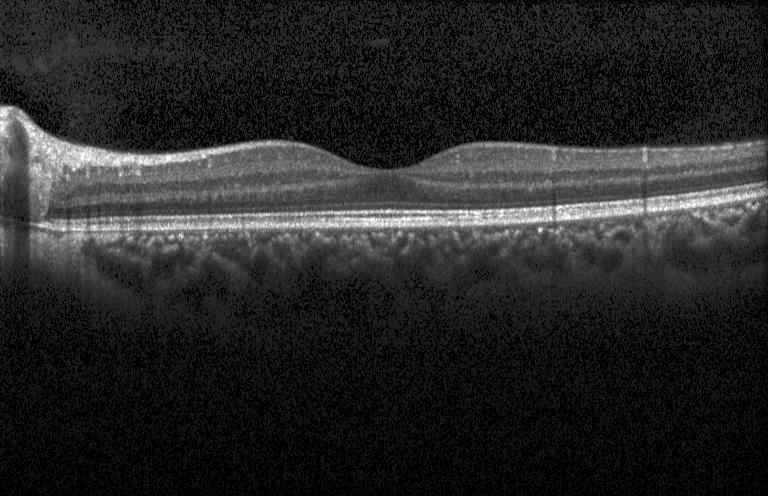 Fovea-centered. Heidelberg Spectralis OCT system. SD-OCT. OCT B-scan. The scan shows no CNV, no DME, and no drusen.